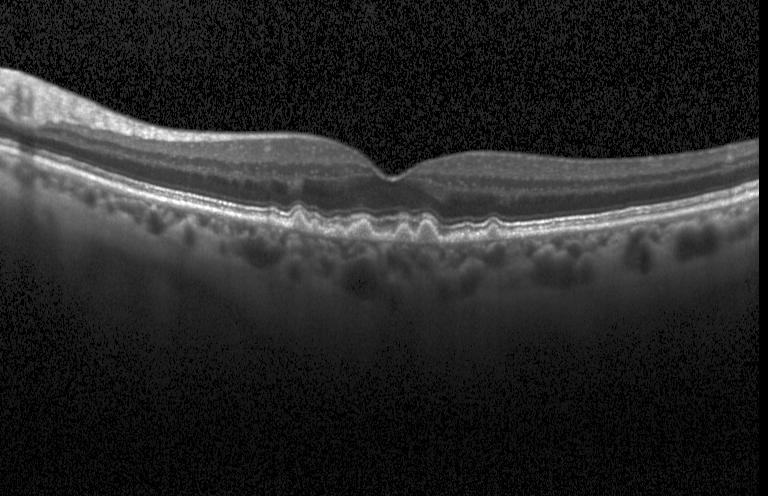

Dx: sub-RPE drusenoid deposits.